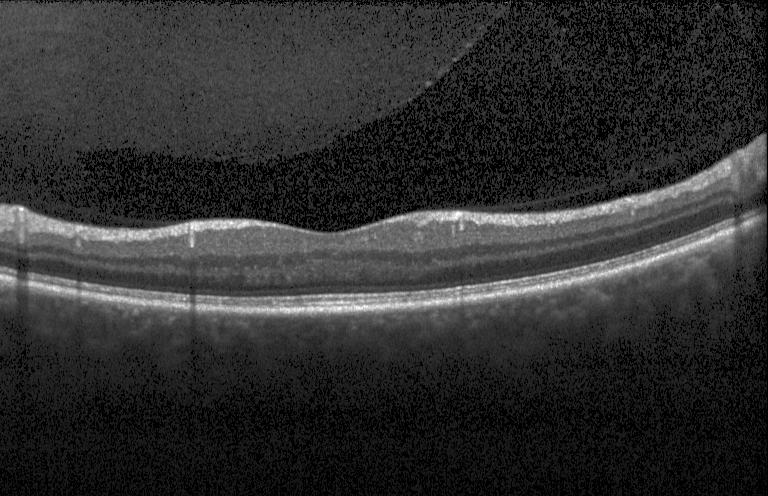 Dx: no choroidal neovascularization, no diabetic macular edema, and no drusen.